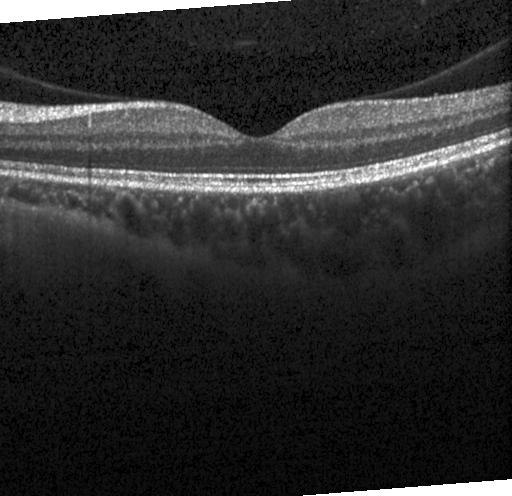

Assessment: no CNV, no DME, and no drusen.